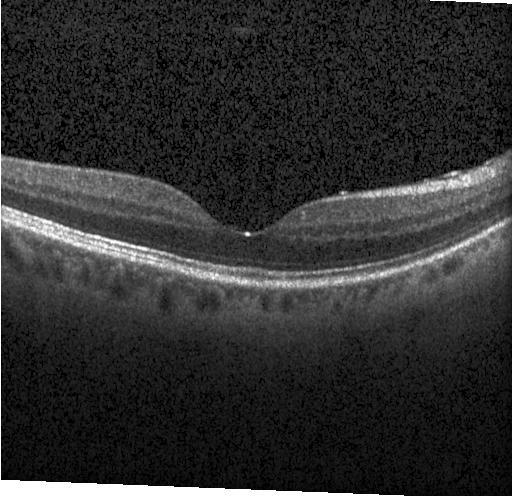 Fovea-centered. Optical coherence tomography B-scan
Dx: no evidence of choroidal neovascularization, diabetic macular edema, or drusen.